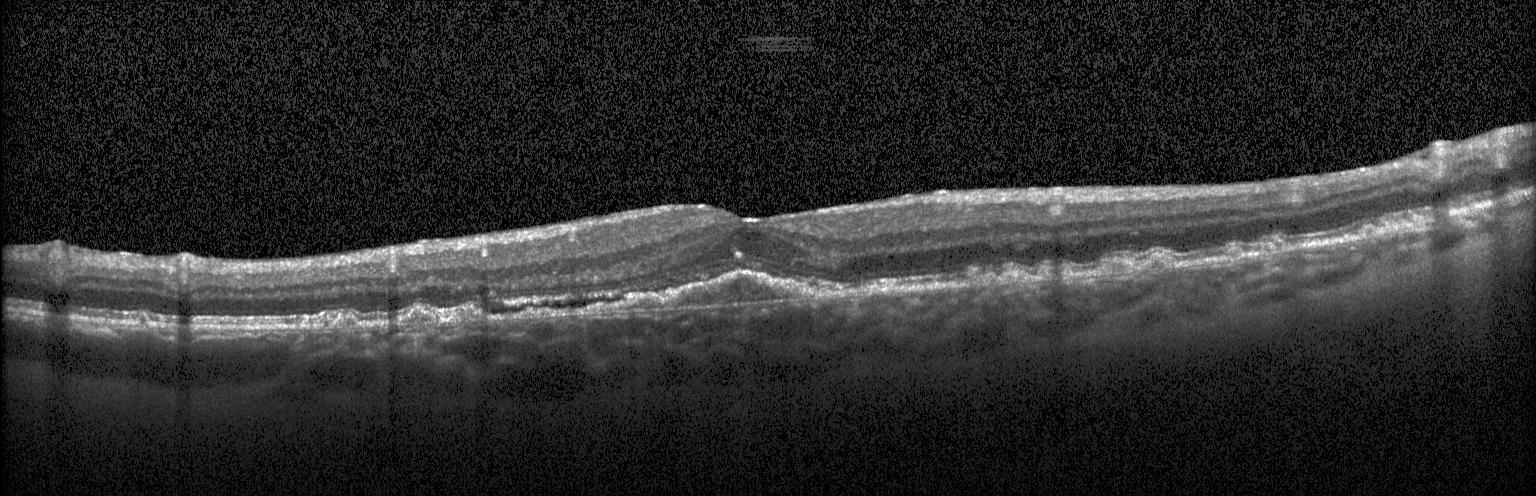 OCT finding: choroidal neovascularization.